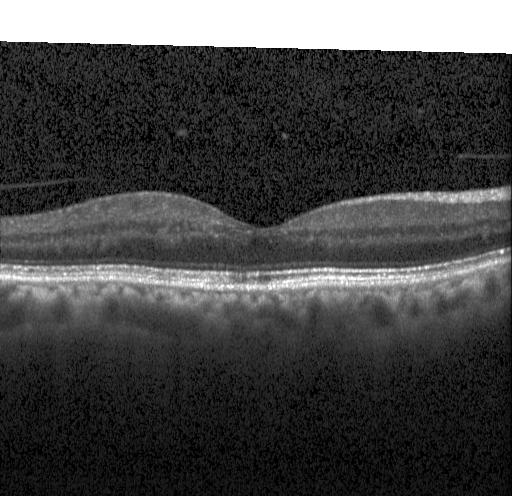
OCT finding: no choroidal neovascularization, diabetic macular edema, or drusen.